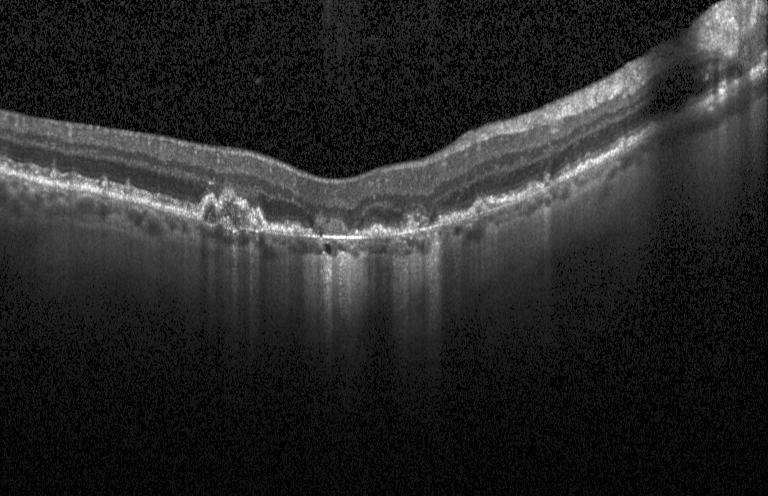

Spectral-domain optical coherence tomography; retinal OCT B-scan; Heidelberg Spectralis OCT system; centered on the fovea.
Impression: a choroidal neovascular membrane.